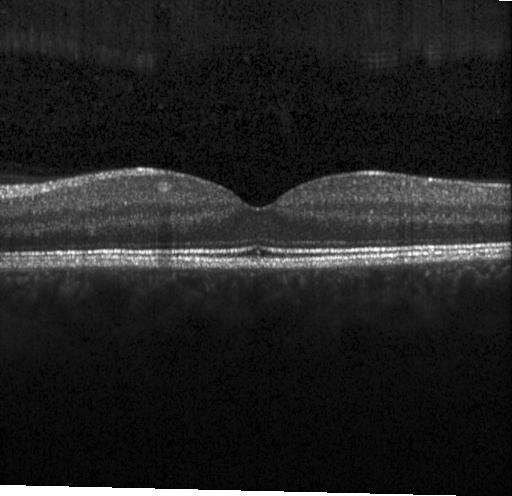

Through the macula · optical coherence tomography B-scan.
Diagnosis: no choroidal neovascularization, diabetic macular edema, or drusen.